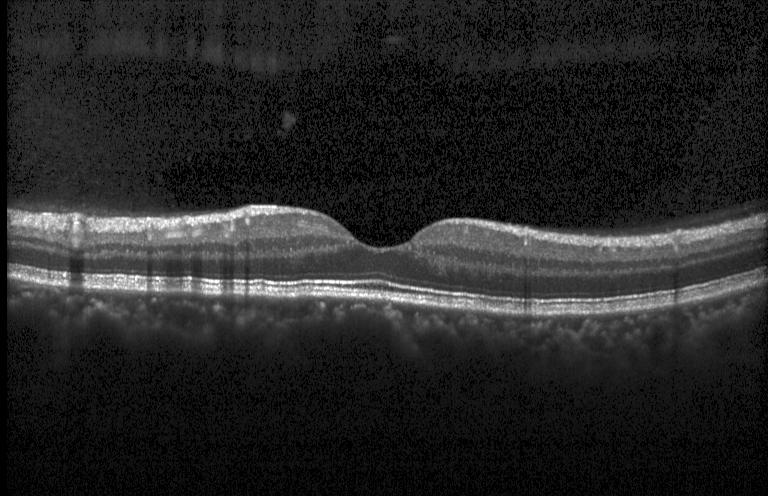
Dx: no evidence of choroidal neovascularization, diabetic macular edema, or drusen.